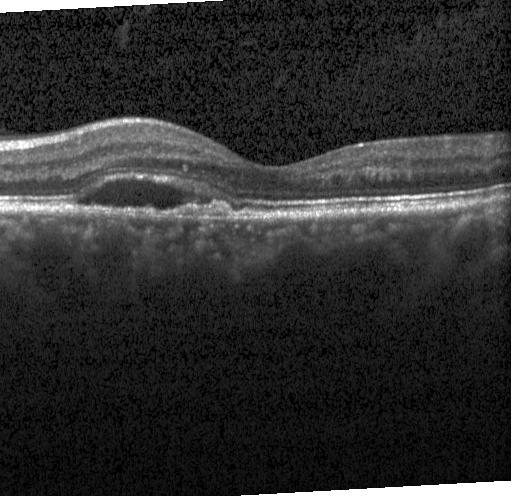
Retinal OCT cross-section; centered on the fovea; spectral-domain optical coherence tomography
Macular OCT: a choroidal neovascular membrane.